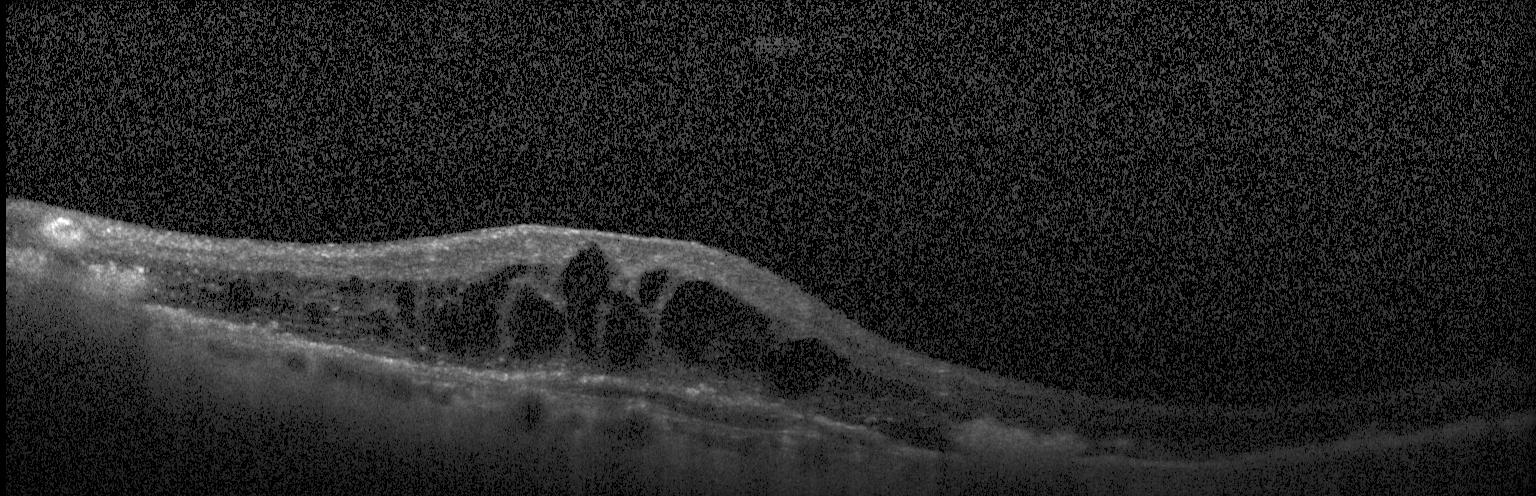 Macular OCT demonstrating choroidal neovascularization (CNV).